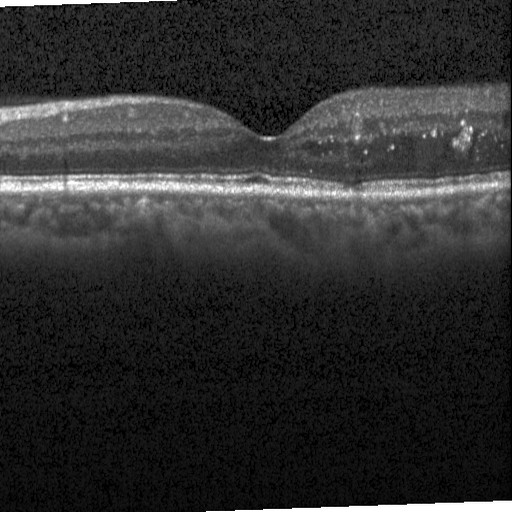
Spectral-domain OCT B-scan: diabetic macular edema (DME).